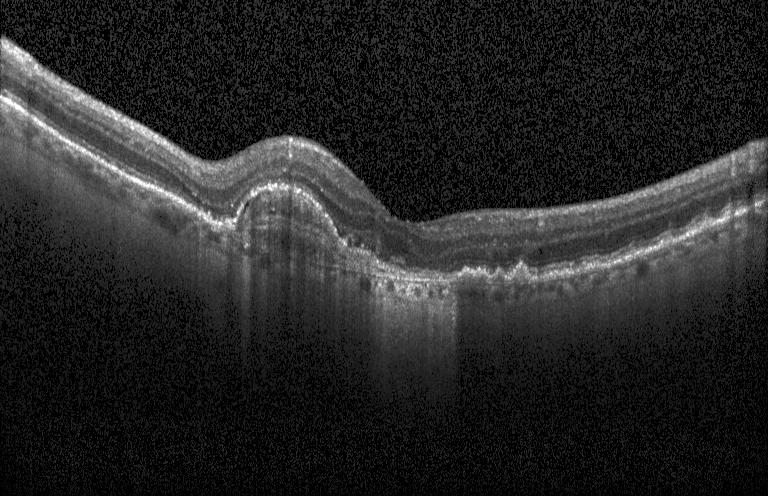
Diagnosis: CNV.